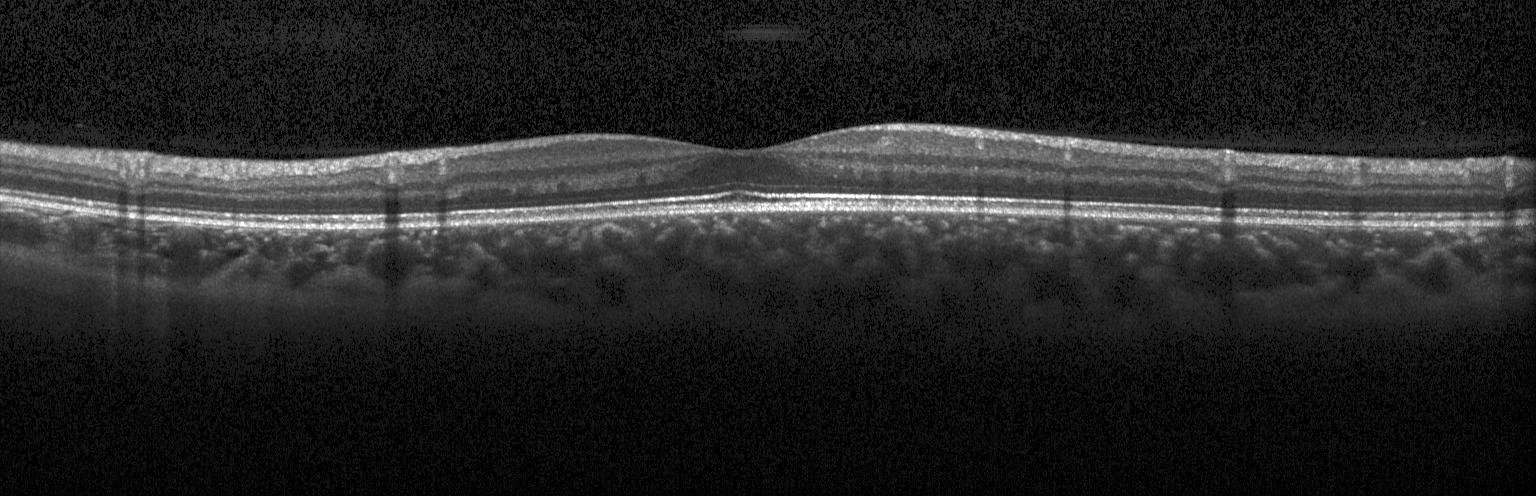 SD-OCT, OCT B-scan, acquired on a Heidelberg Spectralis, macular scan.
Neither choroidal neovascularization, diabetic macular edema, nor drusen.